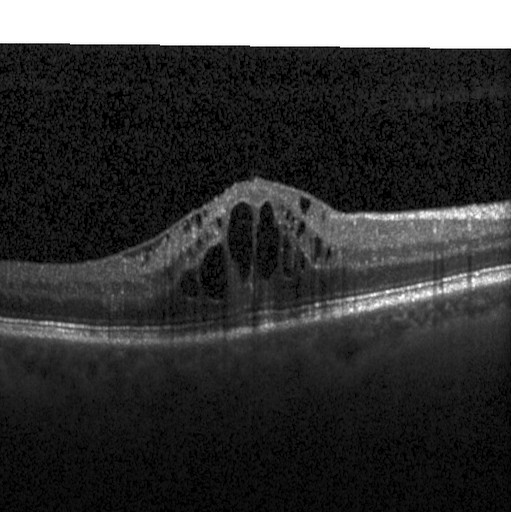

Finding: DME.